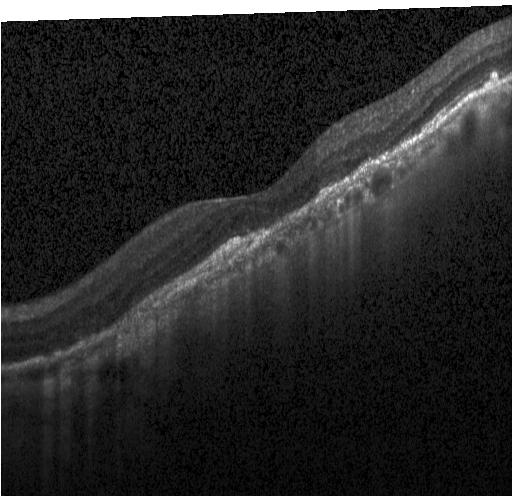

Fovea-centered, optical coherence tomography scan, instrument: Heidelberg Spectralis. Impression: a choroidal neovascular membrane.